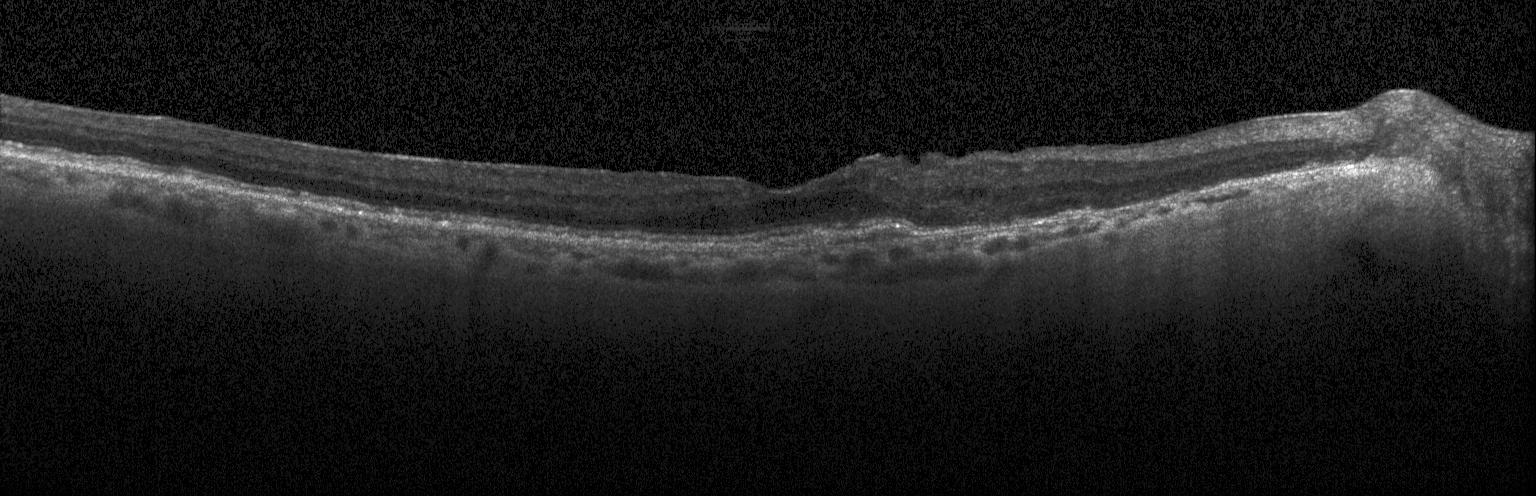

Diagnosis: CNV.